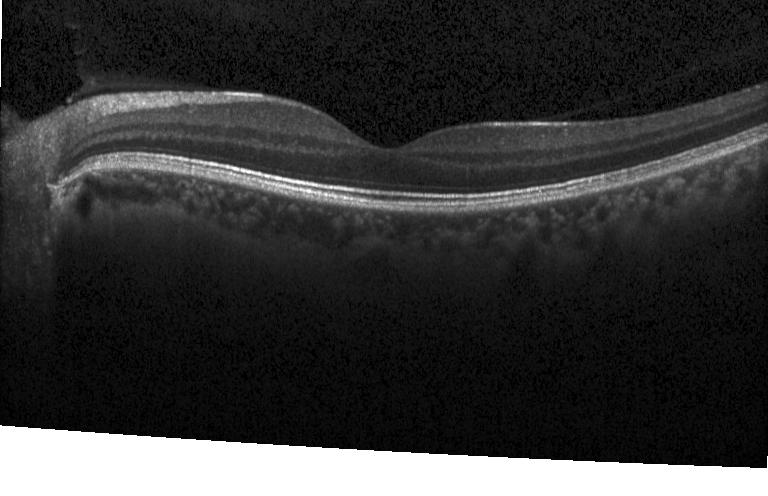

Optical coherence tomography scan — Dx: no CNV, DME, or drusen.